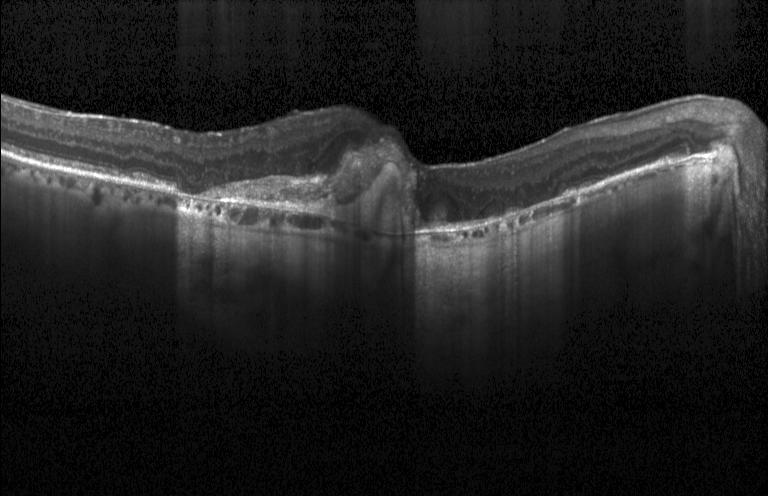
Macular scan. SD-OCT. Optical coherence tomography scan
The scan shows choroidal neovascularization (CNV).